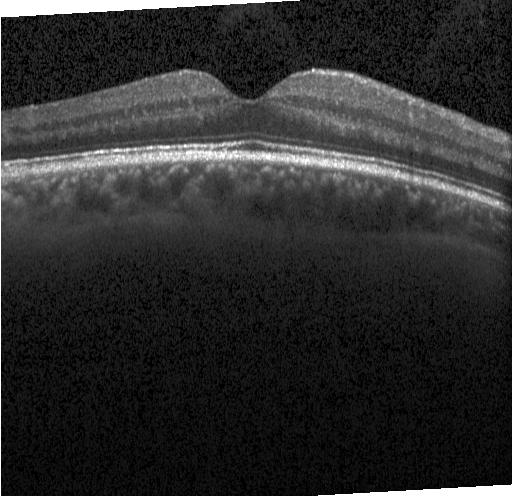

Finding: no evidence of choroidal neovascularization, diabetic macular edema, or drusen.